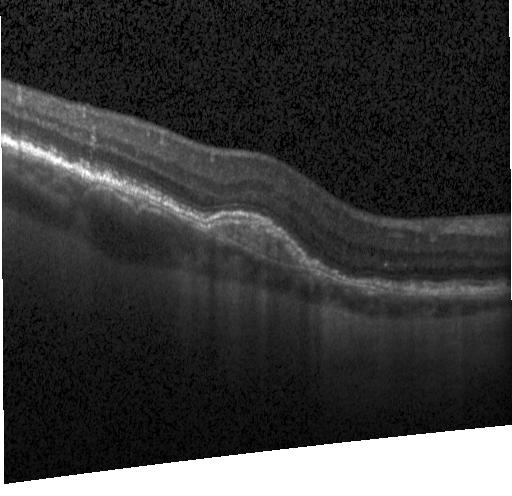
The scan shows choroidal neovascularization (CNV).